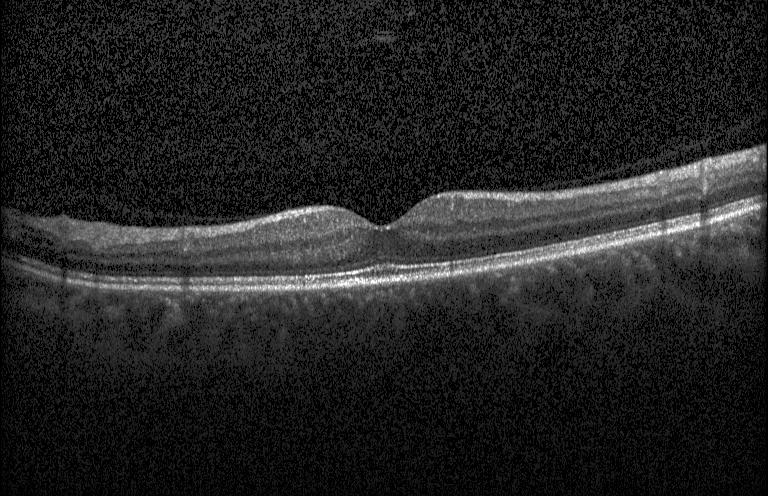
Spectral-domain OCT. Heidelberg Spectralis OCT system. OCT B-scan. Fovea-centered.
Dx: no choroidal neovascularization, diabetic macular edema, or drusen.